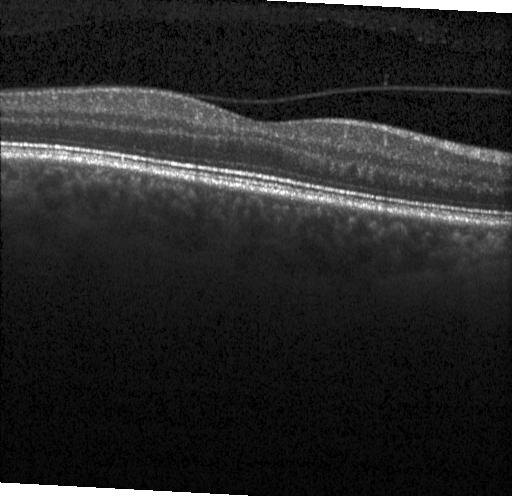 Instrument: Heidelberg Spectralis. OCT B-scan. Impression: neither choroidal neovascularization, diabetic macular edema, nor drusen.